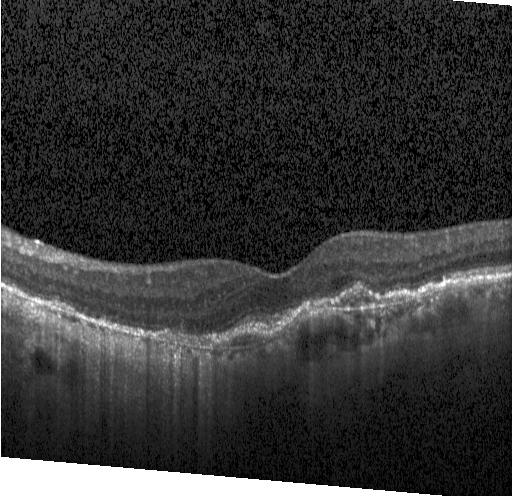 Impression: choroidal neovascularization (CNV).